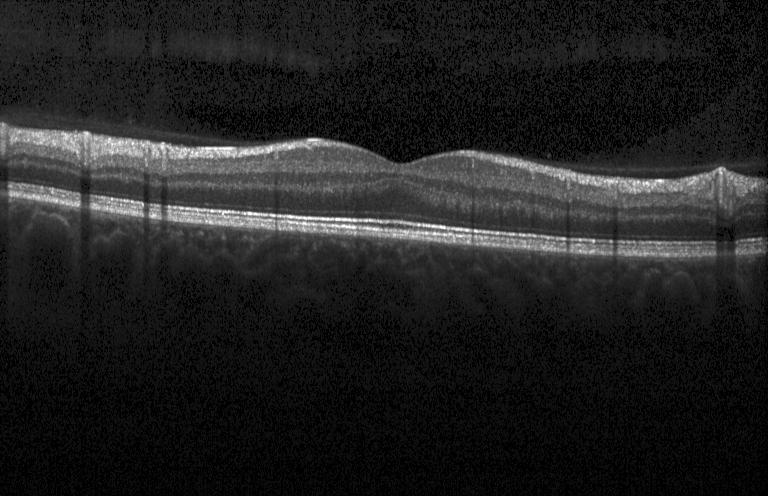

OCT finding: no choroidal neovascularization, diabetic macular edema, or drusen.